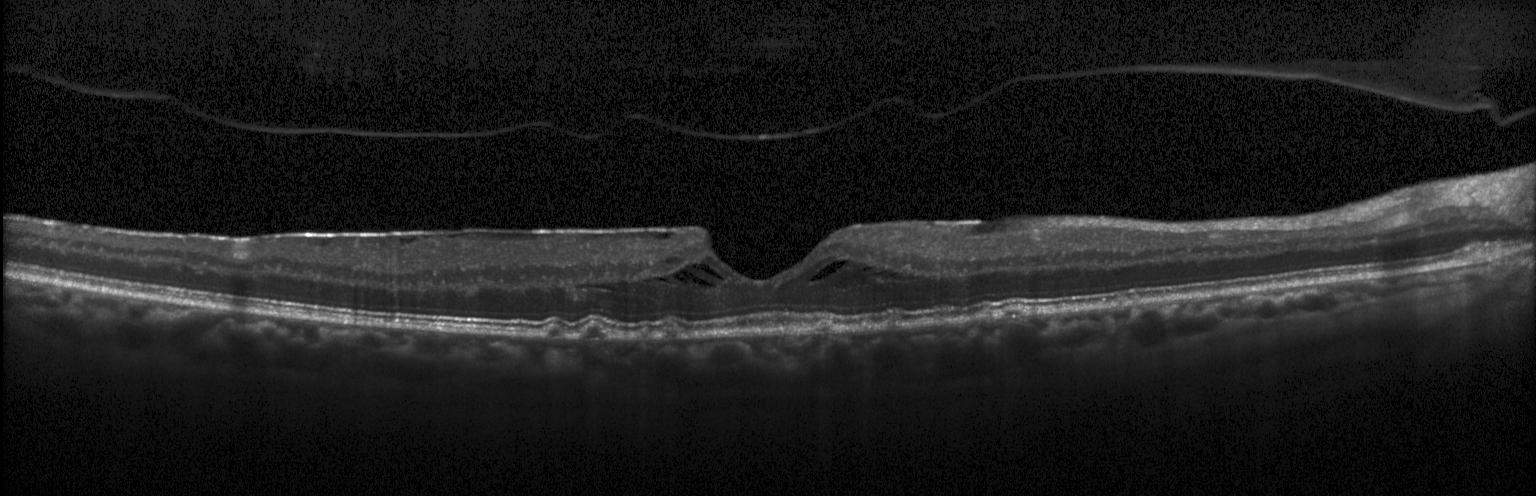
This B-scan demonstrates multiple drusen.